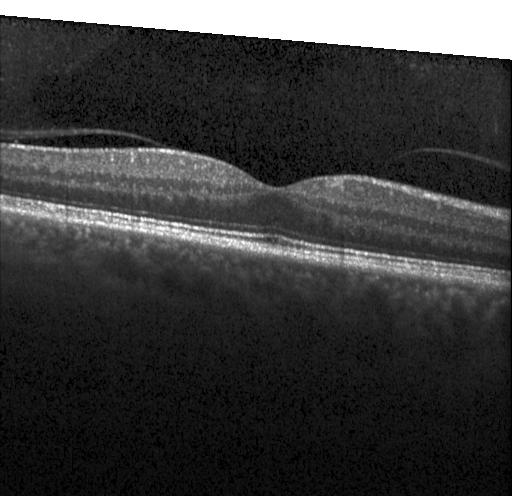 Fovea-centered; SD-OCT; retinal OCT cross-section; Heidelberg Spectralis
The scan shows neither CNV, DME, nor drusen.